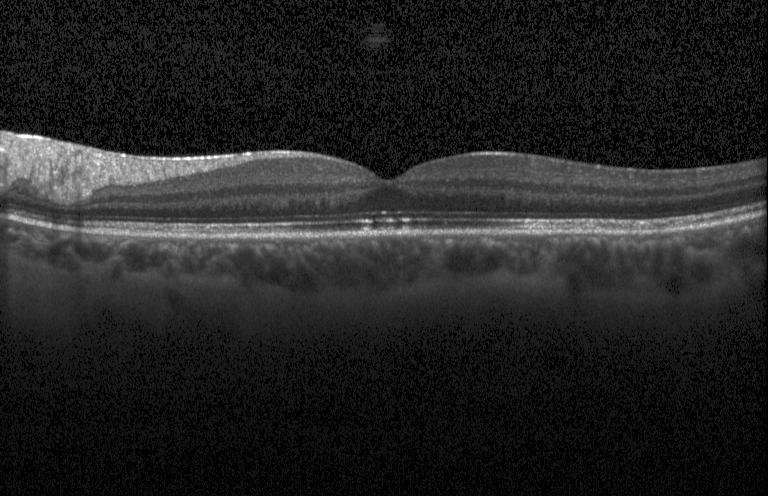

Impression: no CNV, no DME, and no drusen.